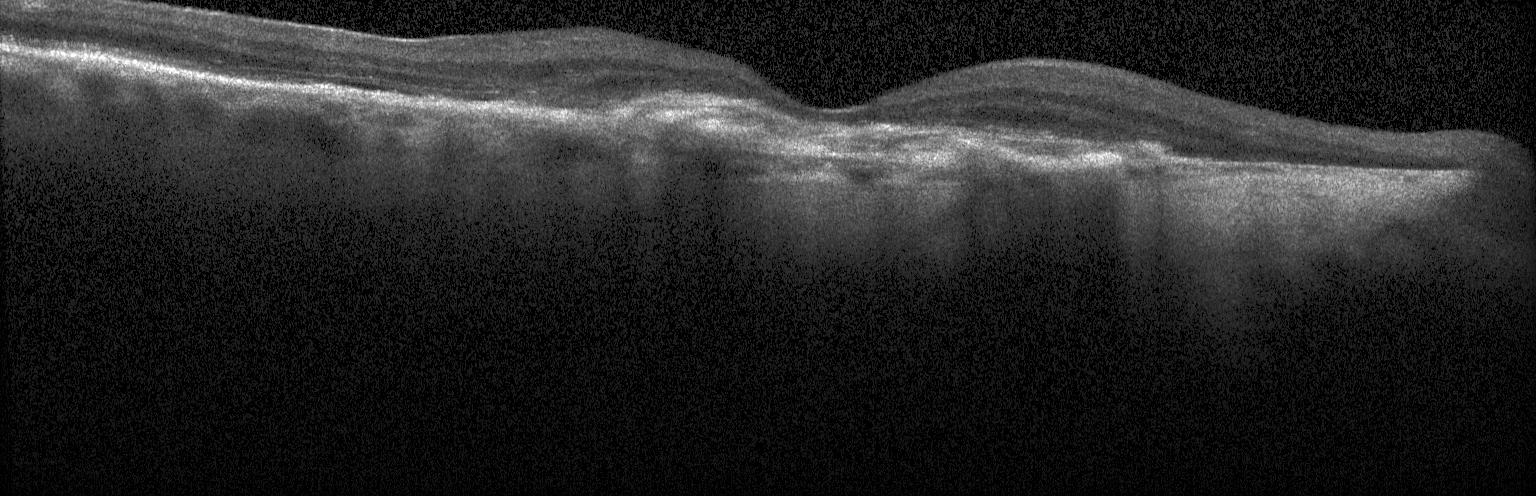
Impression: a choroidal neovascular membrane.